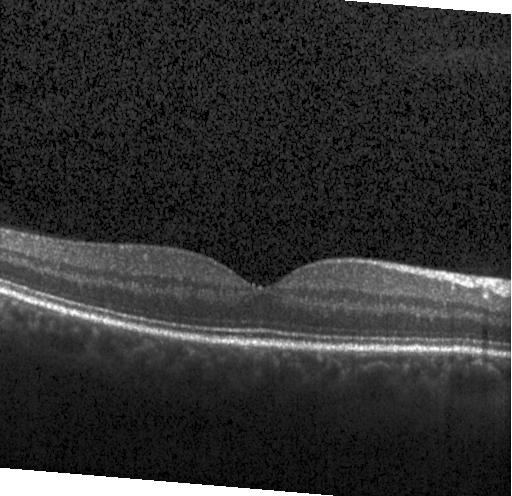

SD-OCT, Heidelberg Spectralis, retinal OCT cross-section. This B-scan demonstrates neither CNV, DME, nor drusen.